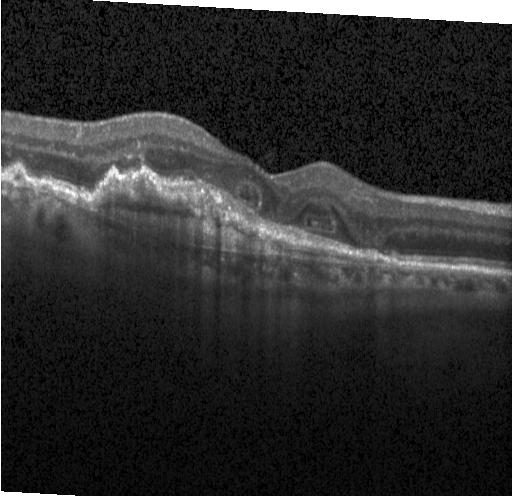
Horizontal scan through the fovea · SD-OCT · OCT line scan · Heidelberg Spectralis.
Dx: a choroidal neovascular membrane.